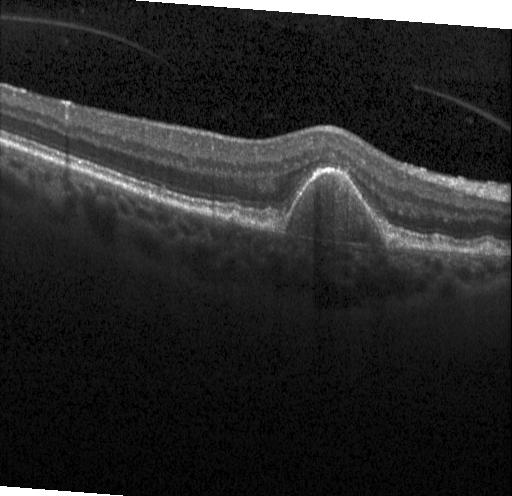

OCT B-scan showing a choroidal neovascular membrane.